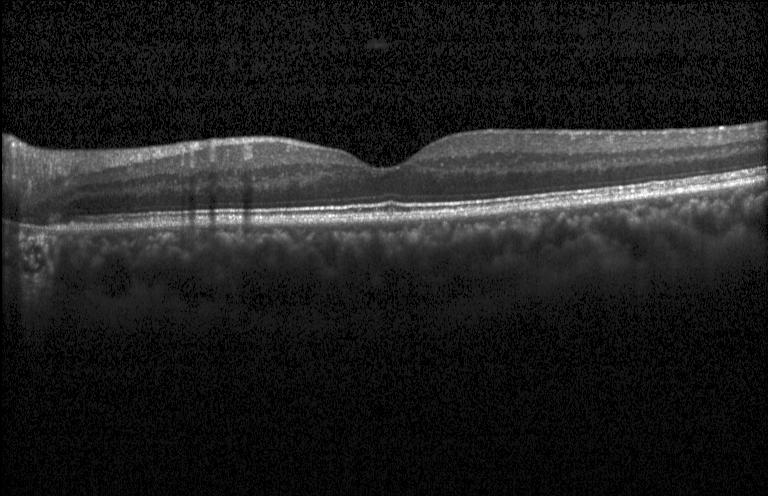
The scan shows no evidence of CNV, DME, or drusen.